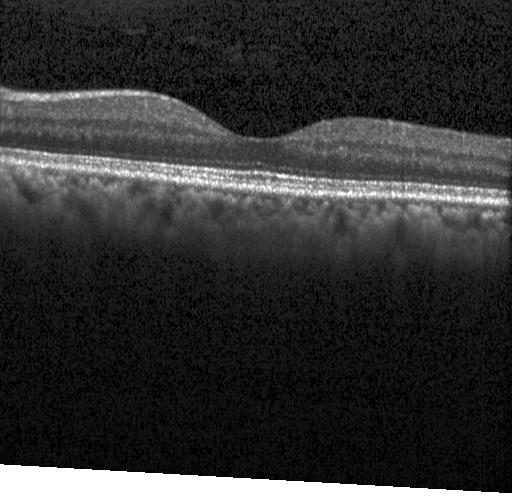

Optical coherence tomography B-scan — The scan shows neither choroidal neovascularization, diabetic macular edema, nor drusen.